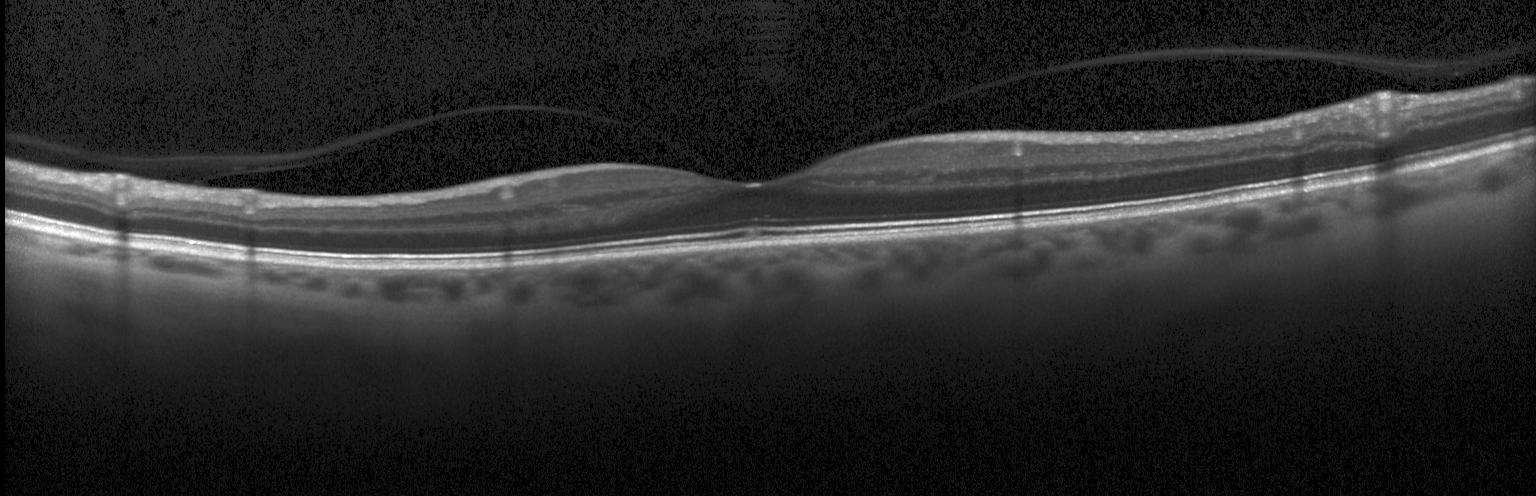

OCT line scan.
Impression: neither choroidal neovascularization, diabetic macular edema, nor drusen.